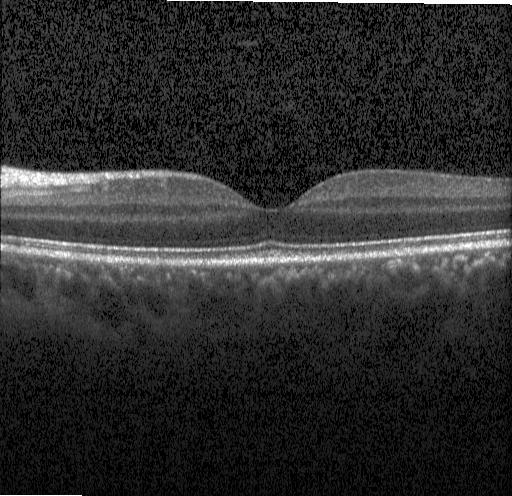
Diagnosis: no choroidal neovascularization, diabetic macular edema, or drusen.